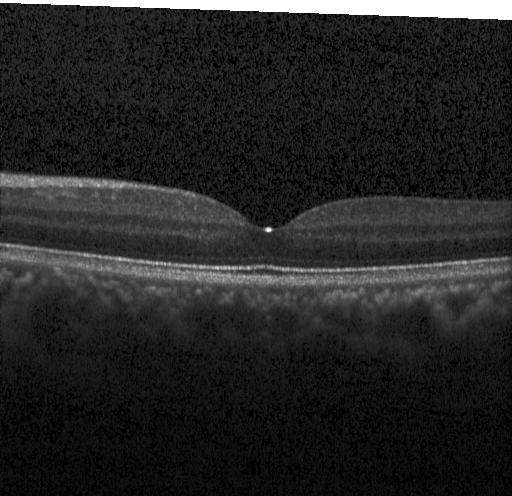

Centered on the fovea. Optical coherence tomography B-scan. Assessment: no evidence of choroidal neovascularization, diabetic macular edema, or drusen.